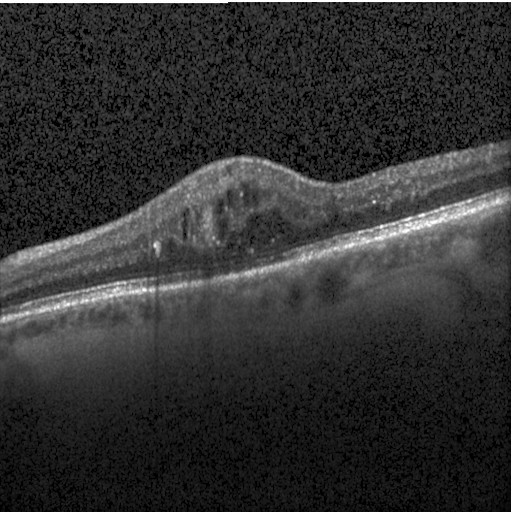
Optical coherence tomography scan, through the macula, instrument: Heidelberg Spectralis, spectral-domain OCT — Assessment: diabetic macular edema (DME).